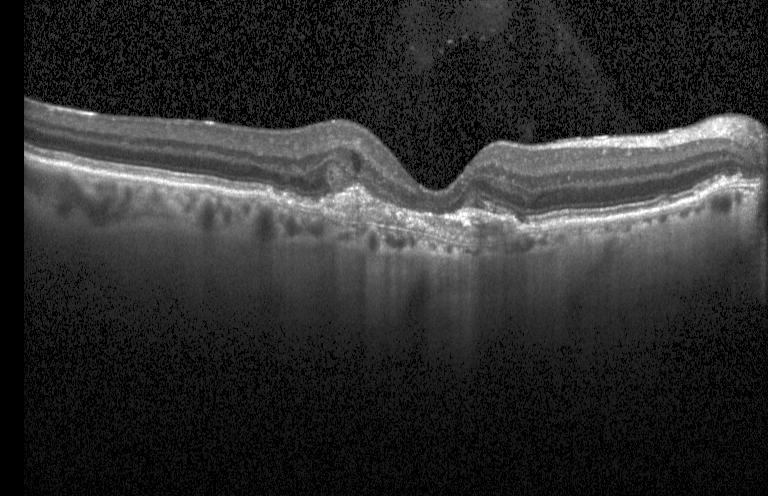
The scan shows a choroidal neovascular membrane.